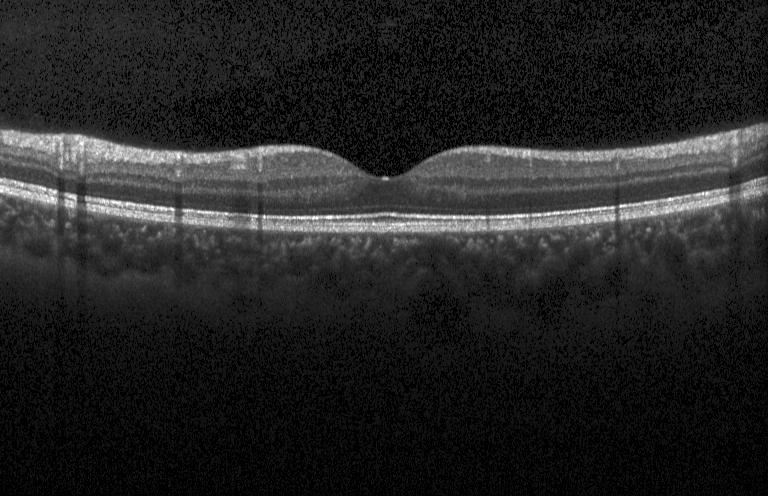
Spectral-domain OCT; through the macula; instrument: Heidelberg Spectralis; OCT line scan. Finding: no evidence of CNV, DME, or drusen.